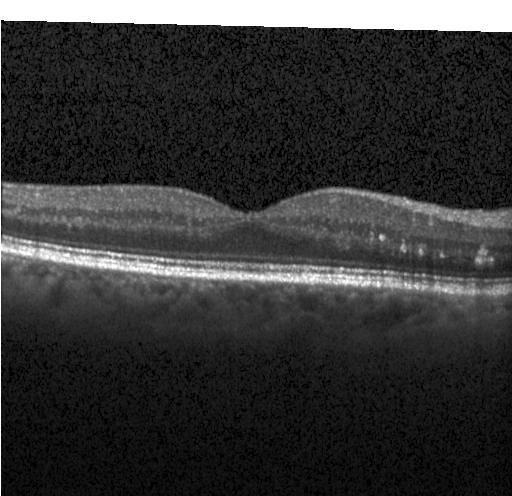 Spectral-domain OCT. OCT B-scan. This B-scan demonstrates no choroidal neovascularization, no diabetic macular edema, and no drusen.